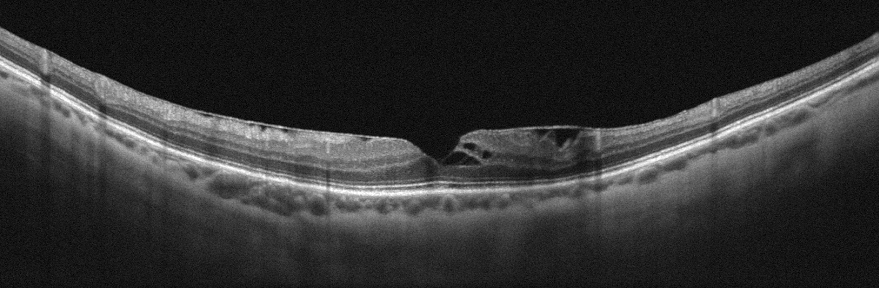 Left eye, instrument: Optovue Avanti RTVue XR, retinal OCT cross-section, macular scan
OCT finding: vitreomacular interface disease (VID).